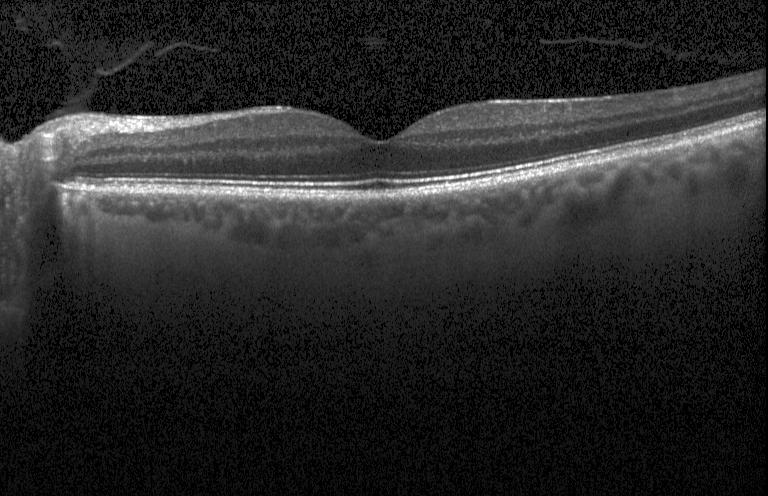
Spectral-domain optical coherence tomography; optical coherence tomography scan; Heidelberg Spectralis; centered on the fovea.
Finding: no CNV, DME, or drusen.